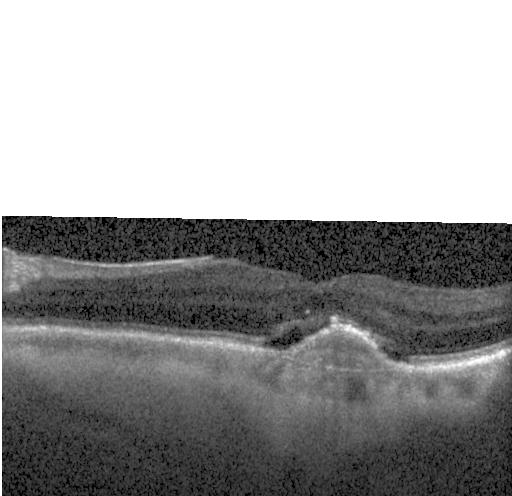
Optical coherence tomography B-scan; Heidelberg Spectralis OCT system; SD-OCT; fovea-centered. CNV.